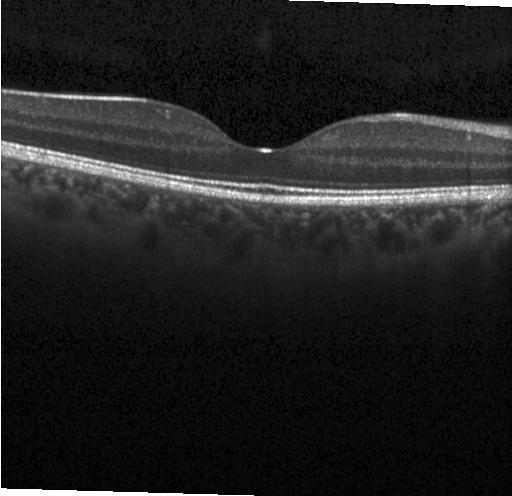

Finding: no CNV, no DME, and no drusen.